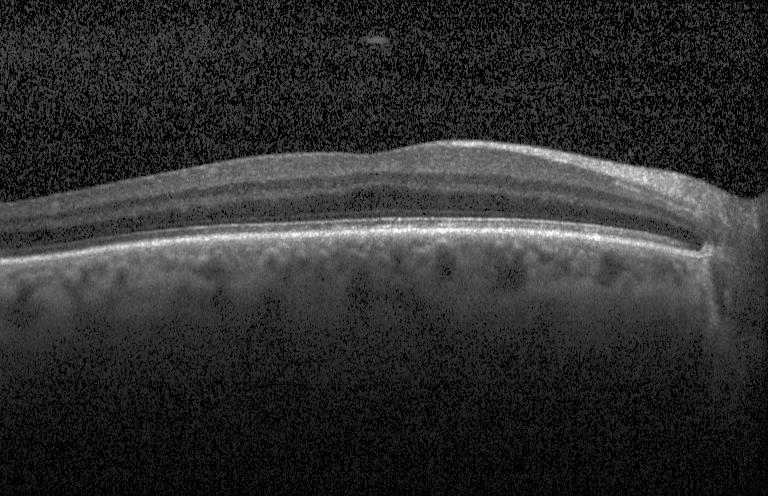

The scan shows no evidence of choroidal neovascularization, diabetic macular edema, or drusen.